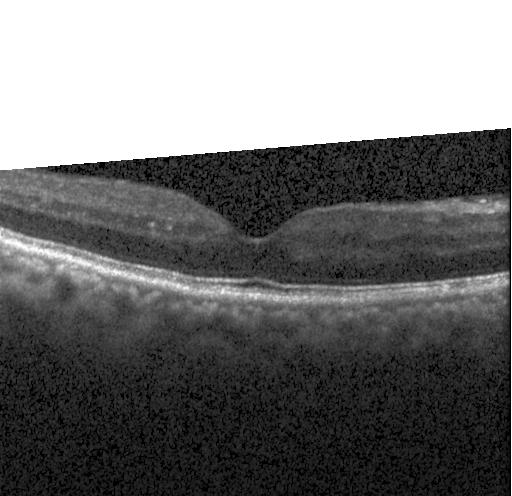

Optical coherence tomography scan.
Impression: no choroidal neovascularization, diabetic macular edema, or drusen.